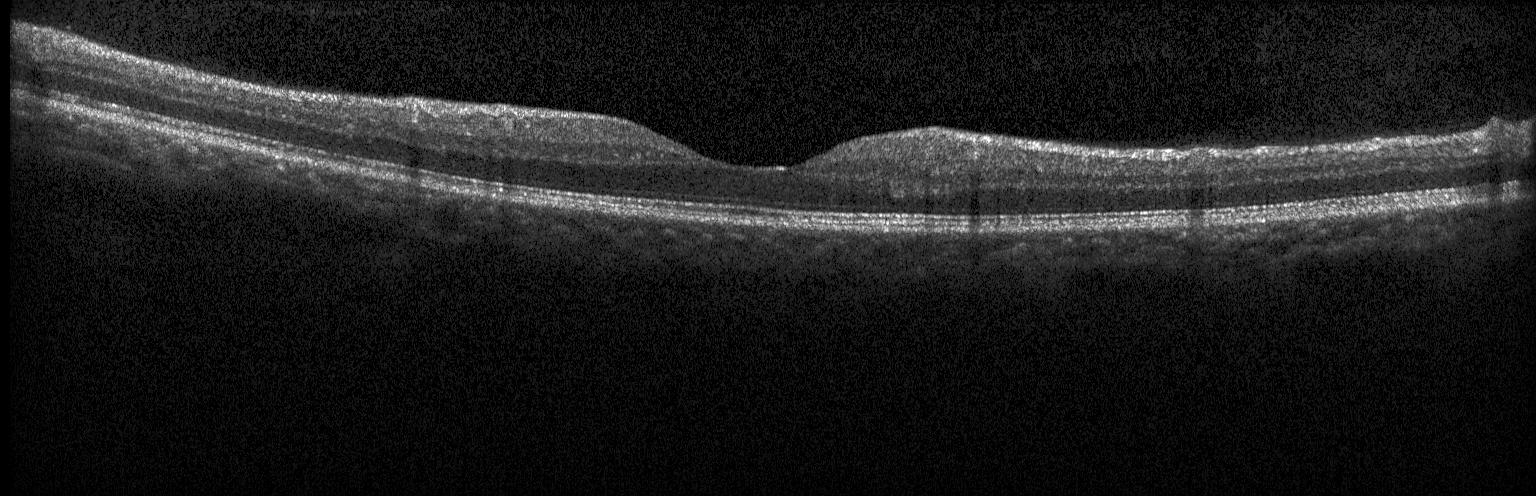
Optical coherence tomography scan, acquired on a Heidelberg Spectralis, SD-OCT. Neither CNV, DME, nor drusen.